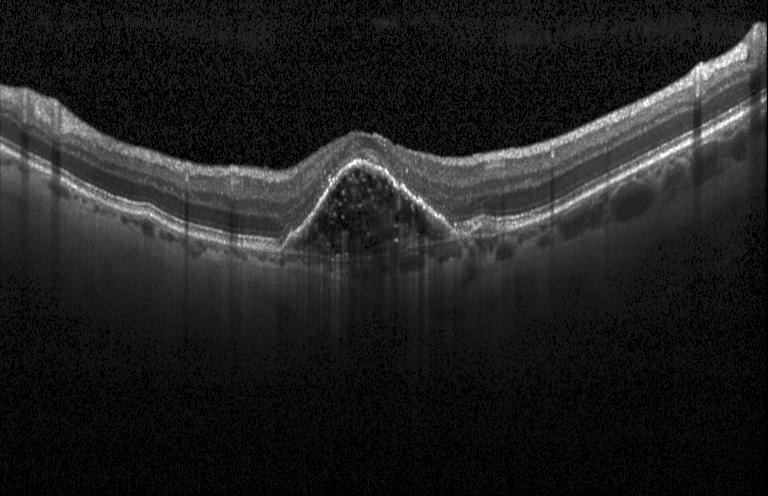 Fovea-centered, spectral-domain optical coherence tomography, Heidelberg Spectralis, optical coherence tomography B-scan
This B-scan demonstrates a choroidal neovascular membrane.